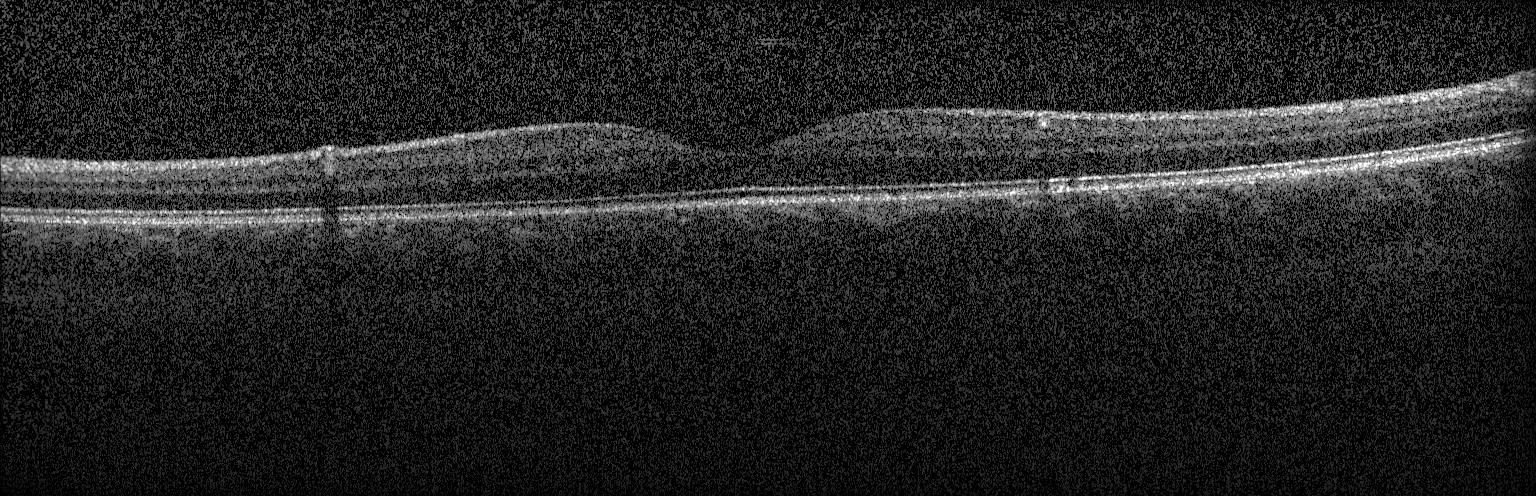
OCT scan showing no choroidal neovascularization, no diabetic macular edema, and no drusen.